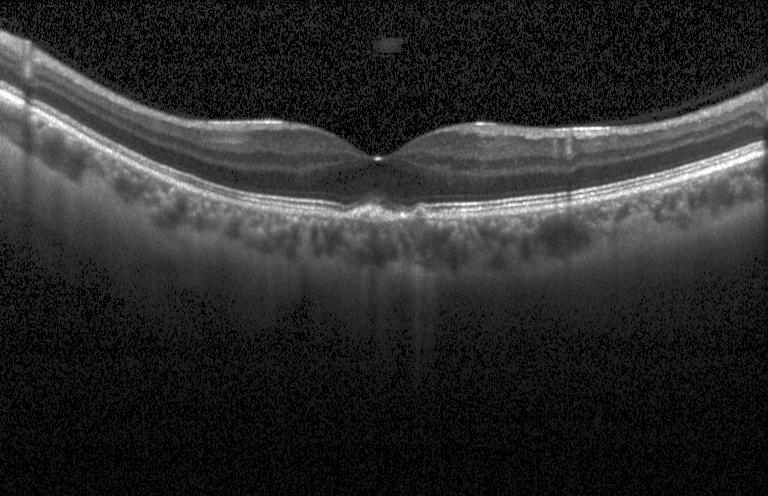
Retinal OCT cross-section. Impression: choroidal neovascularization.